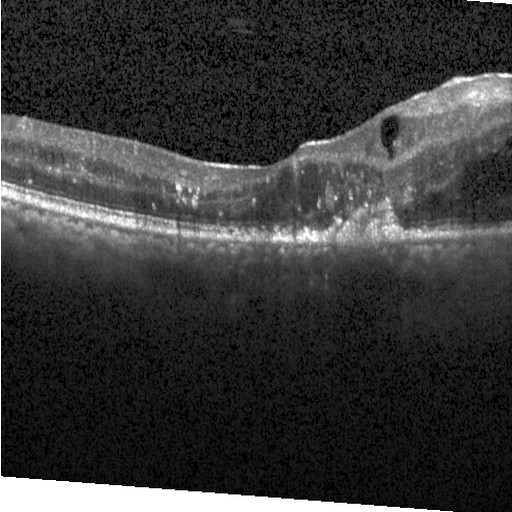 Instrument: Heidelberg Spectralis, horizontal scan through the fovea, optical coherence tomography scan. Dx: DME.